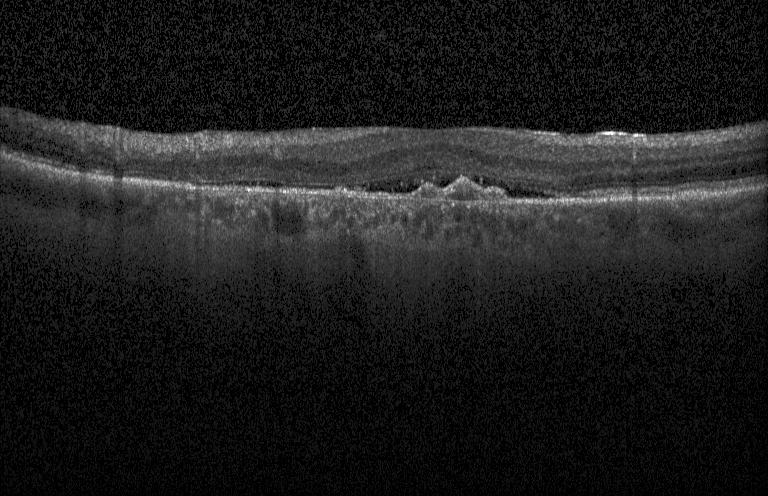 OCT B-scan
The scan shows a choroidal neovascular membrane.